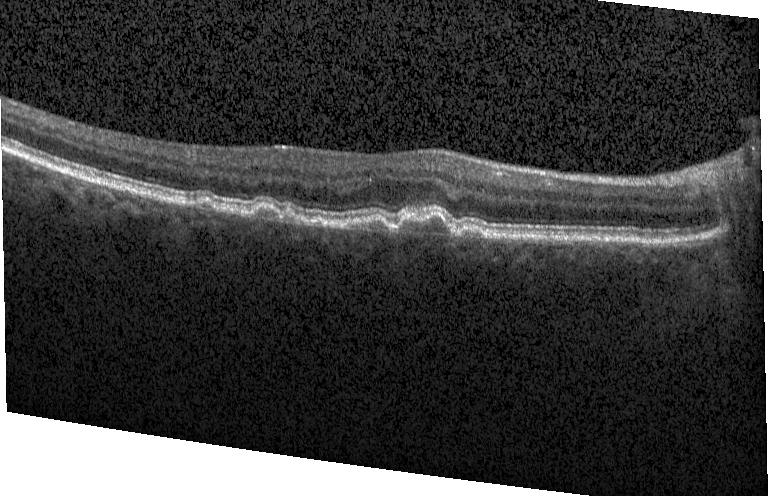 Drusen.